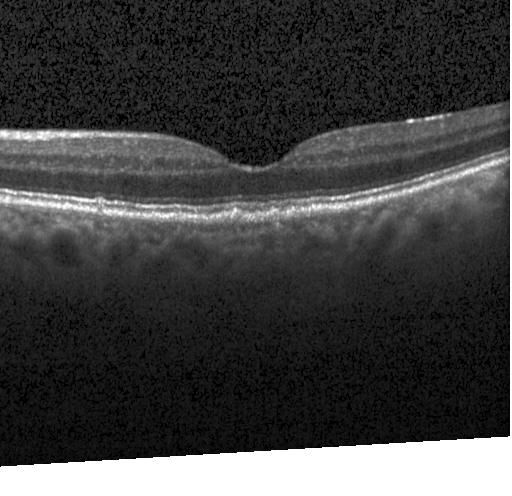
Spectral-domain optical coherence tomography. OCT line scan
Drusen.